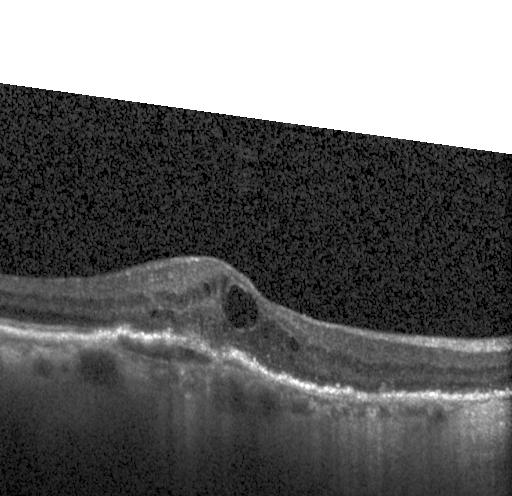

Spectral-domain optical coherence tomography · Heidelberg Spectralis · optical coherence tomography B-scan · fovea-centered — Diagnosis: a choroidal neovascular membrane.